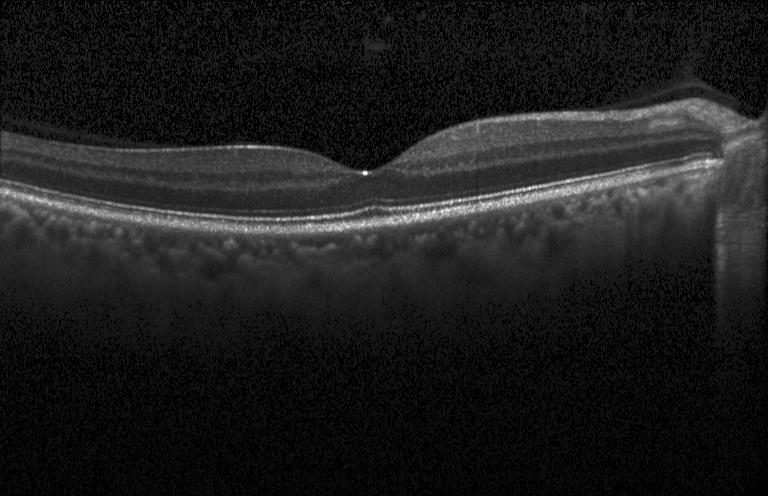 OCT B-scan.
This B-scan demonstrates neither CNV, DME, nor drusen.